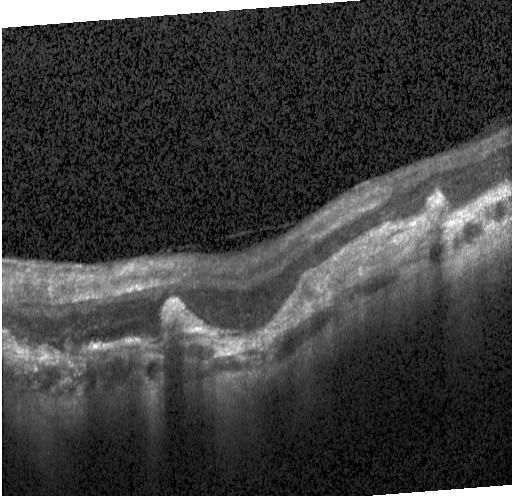 A choroidal neovascular membrane.